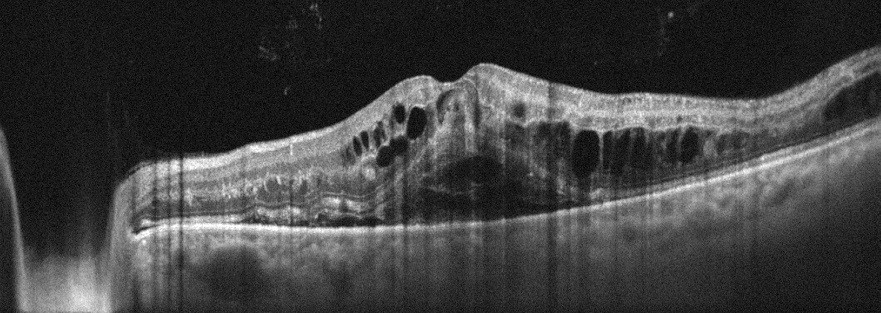

Impression: retinal vein occlusion.